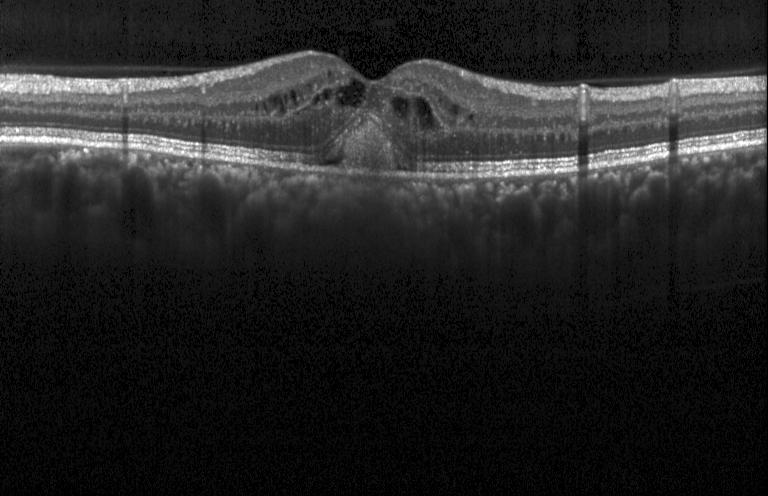 OCT line scan; acquired on a Heidelberg Spectralis; spectral-domain OCT — Diagnosis: choroidal neovascularization.